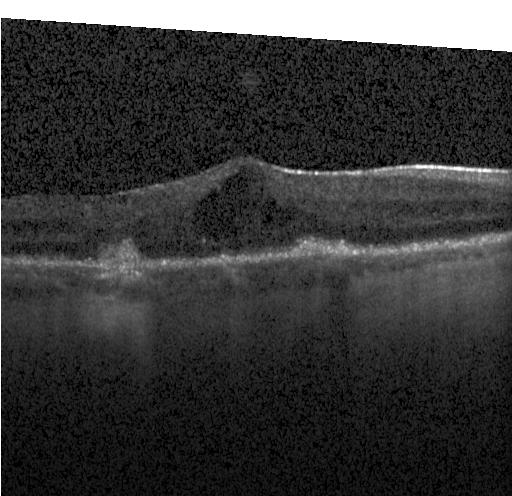 Optical coherence tomography B-scan. OCT finding: a choroidal neovascular membrane.